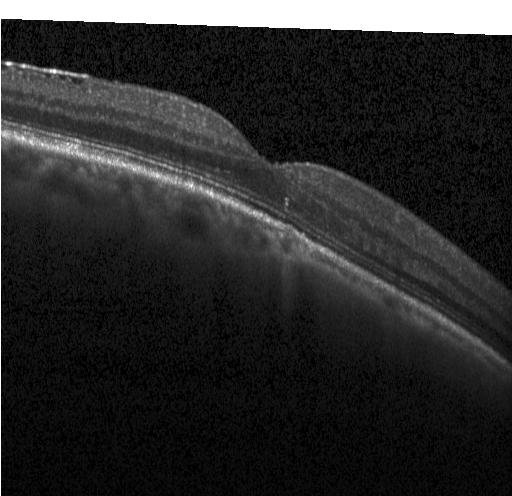 OCT line scan; spectral-domain OCT — Impression: no CNV, DME, or drusen.